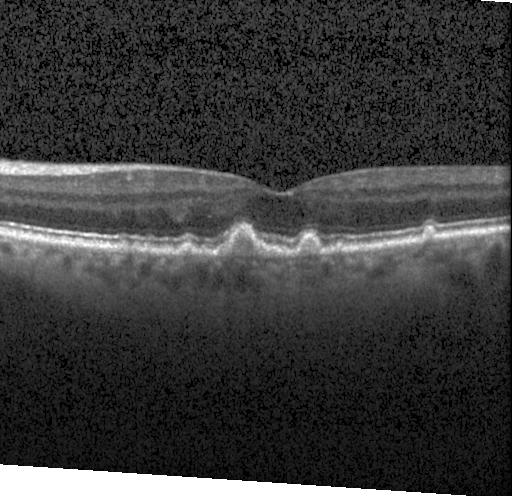
Spectral-domain optical coherence tomography, retinal OCT B-scan, Heidelberg Spectralis.
Dx: drusen.